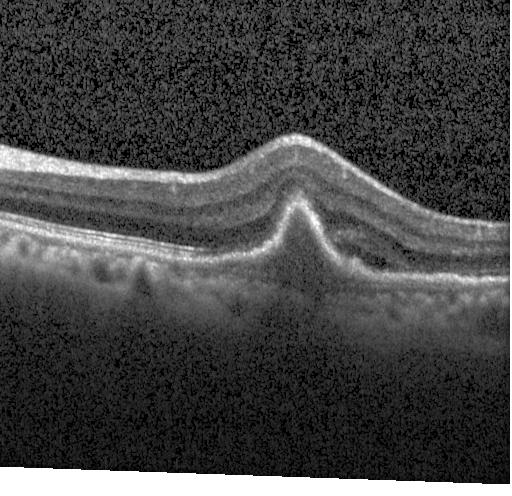
OCT line scan
Impression: a choroidal neovascular membrane.